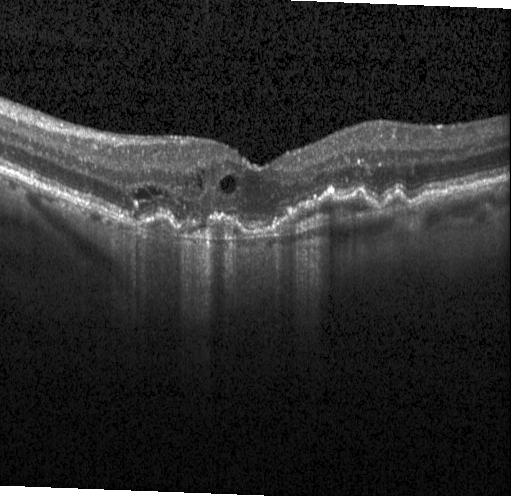

Horizontal scan through the fovea; instrument: Heidelberg Spectralis; optical coherence tomography scan. Impression: a choroidal neovascular membrane.